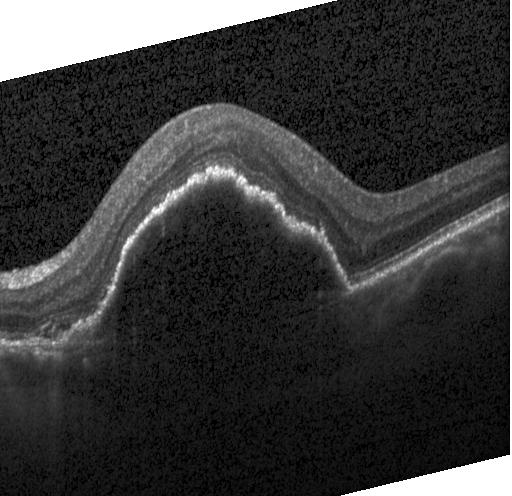 Impression: choroidal neovascularization.